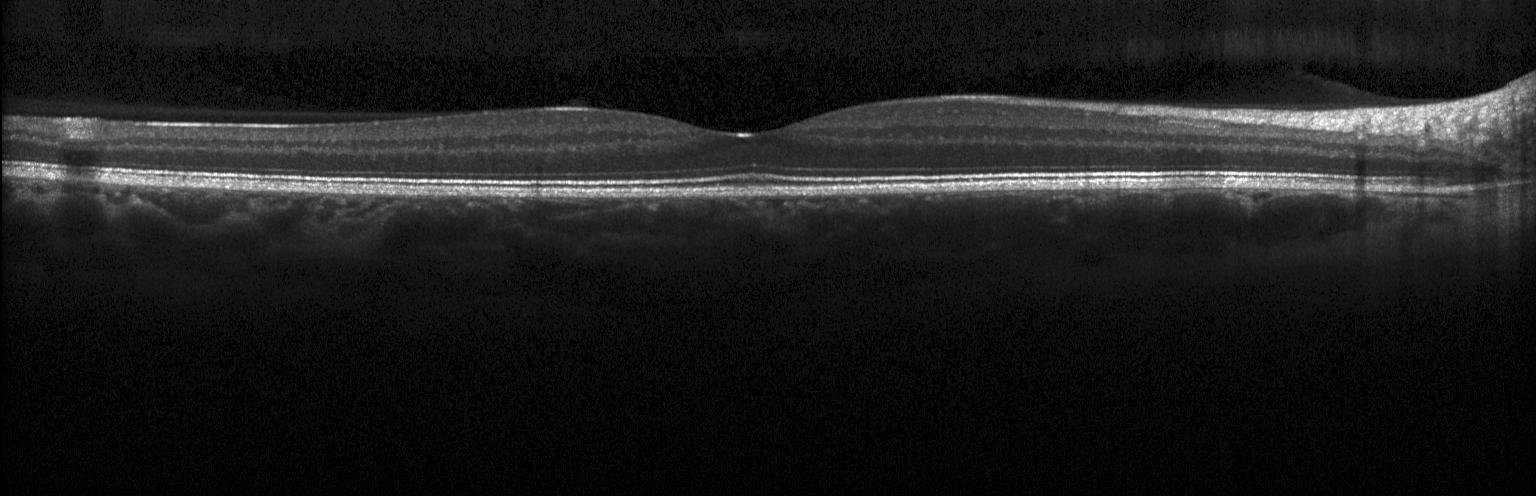
Dx: no evidence of choroidal neovascularization, diabetic macular edema, or drusen.